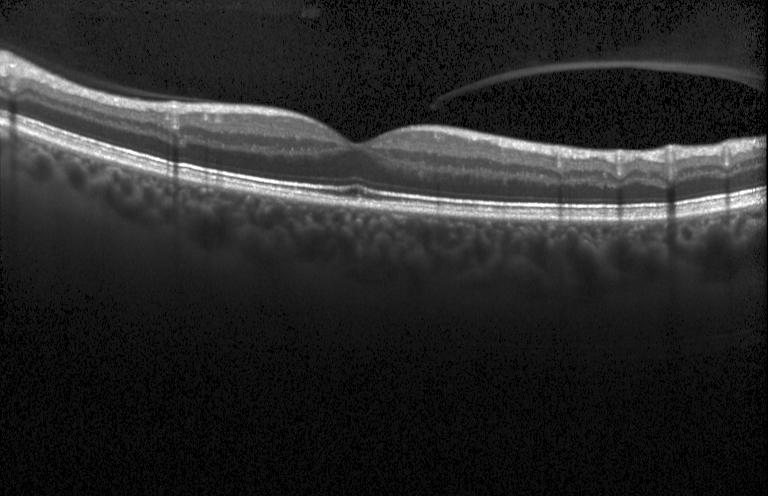 Spectral-domain optical coherence tomography. OCT line scan. Heidelberg Spectralis OCT system. Through the macula — Diagnosis: no choroidal neovascularization, diabetic macular edema, or drusen.